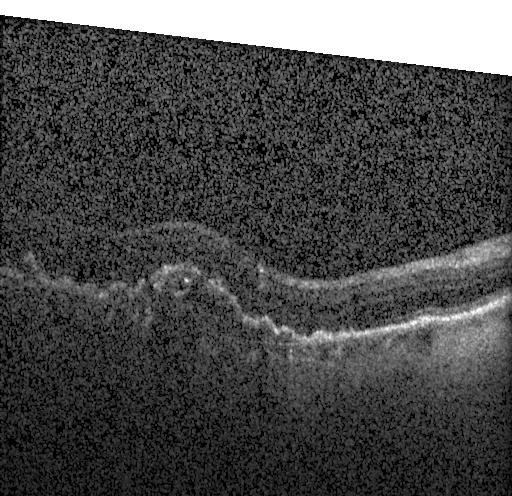 SD-OCT. Instrument: Heidelberg Spectralis. Through the macula. Optical coherence tomography B-scan
Finding: a choroidal neovascular membrane.